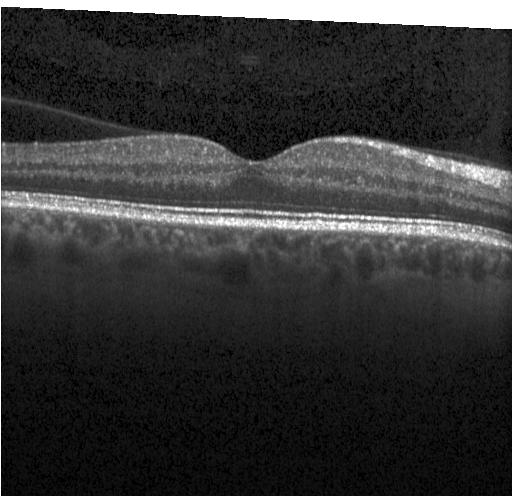 Macular OCT: no choroidal neovascularization, no diabetic macular edema, and no drusen.